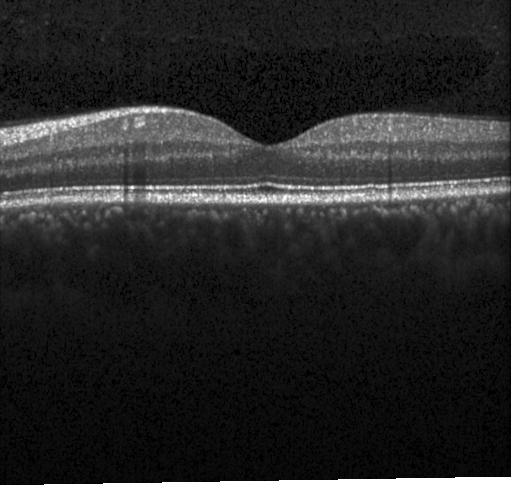
Optical coherence tomography scan
Dx: no CNV, DME, or drusen.